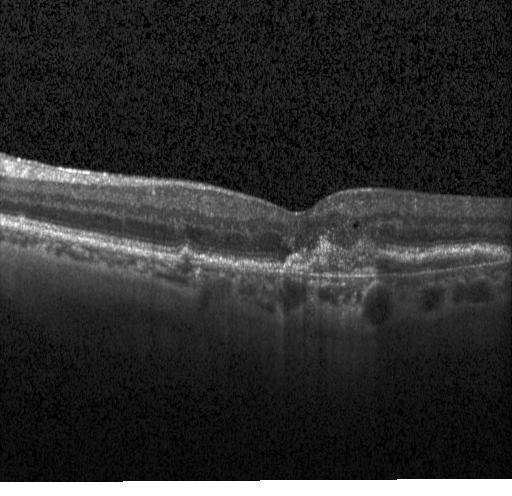
Retinal OCT B-scan — Finding: a choroidal neovascular membrane.